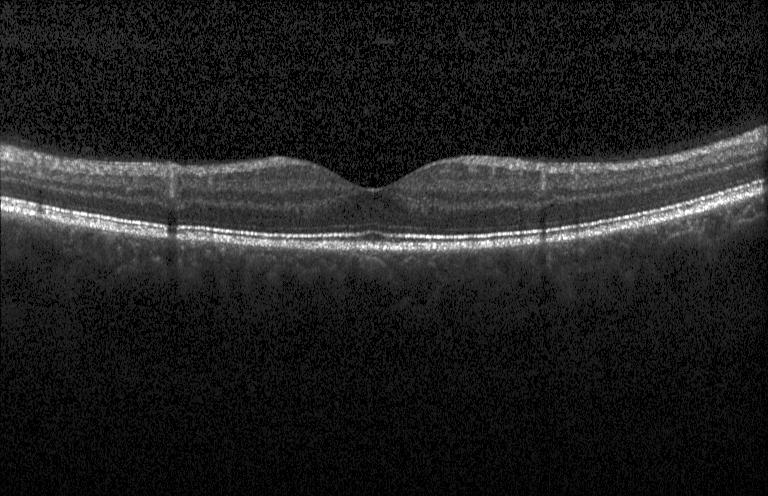

OCT line scan
Assessment: no choroidal neovascularization, no diabetic macular edema, and no drusen.